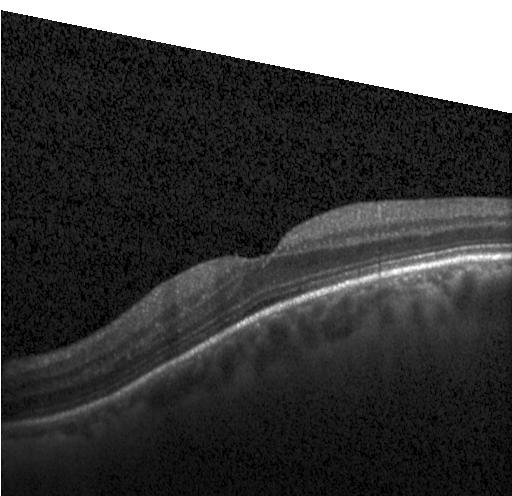 Assessment: neither choroidal neovascularization, diabetic macular edema, nor drusen.